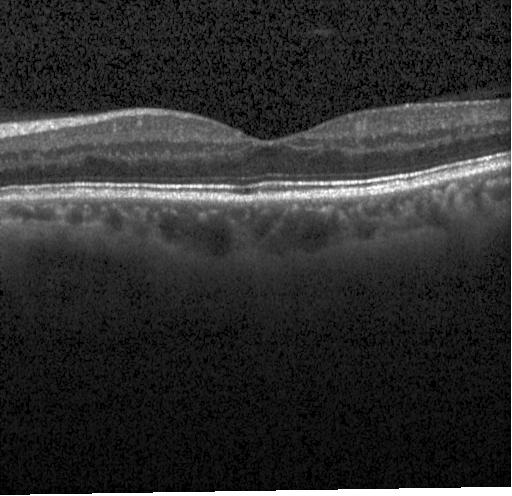

Macular OCT demonstrating no choroidal neovascularization, no diabetic macular edema, and no drusen.